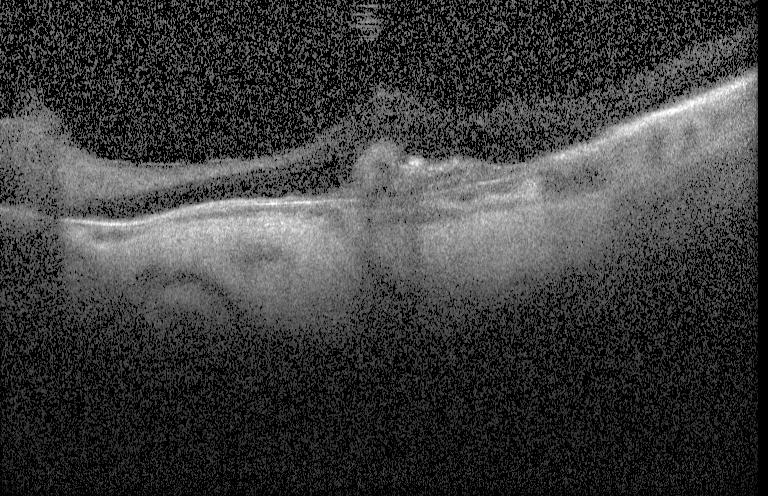 Instrument: Heidelberg Spectralis; retinal OCT cross-section.
Assessment: choroidal neovascularization.